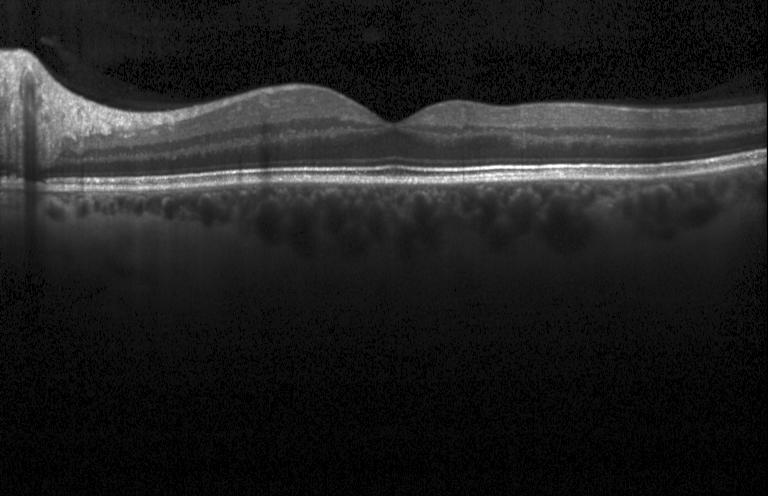 Retinal OCT cross-section showing no choroidal neovascularization, diabetic macular edema, or drusen.